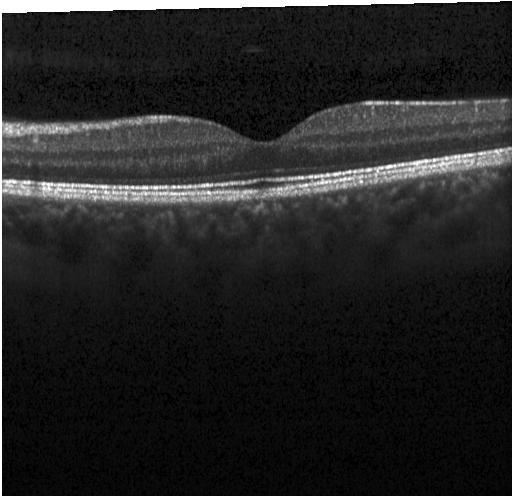 Spectral-domain optical coherence tomography · Heidelberg Spectralis OCT system · retinal OCT cross-section — The scan shows no CNV, DME, or drusen.